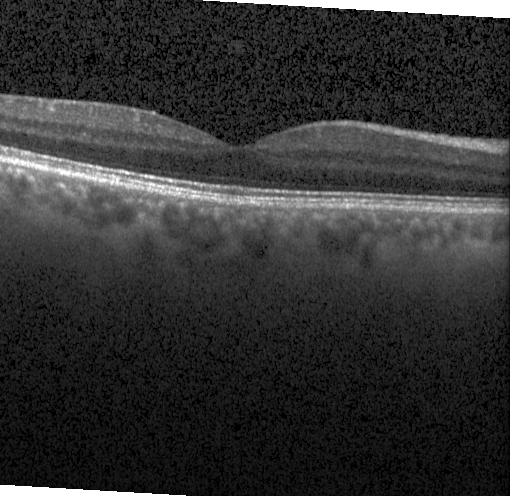

This B-scan demonstrates no choroidal neovascularization, diabetic macular edema, or drusen.